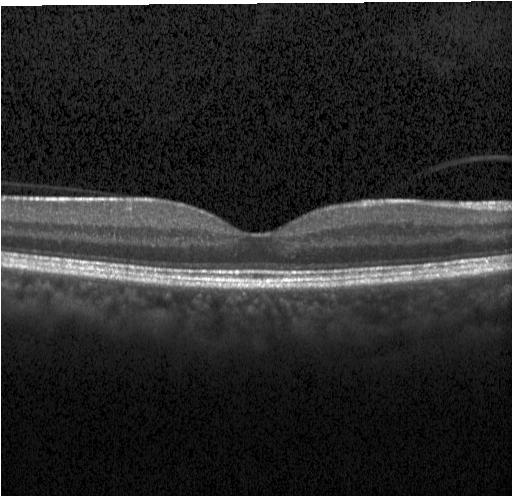 OCT scan showing neither choroidal neovascularization, diabetic macular edema, nor drusen.